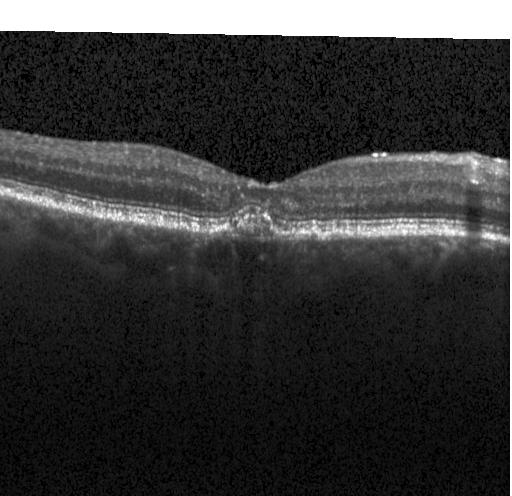
The scan shows drusen.